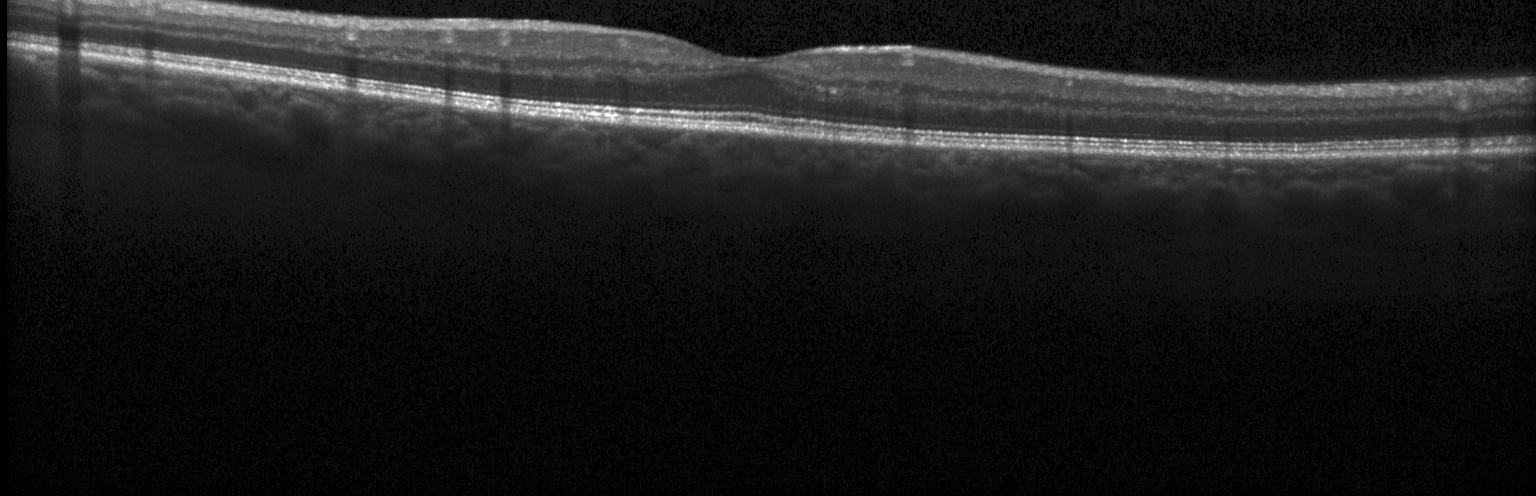

Instrument: Heidelberg Spectralis; macular scan; OCT B-scan.
Macular OCT: no choroidal neovascularization, no diabetic macular edema, and no drusen.